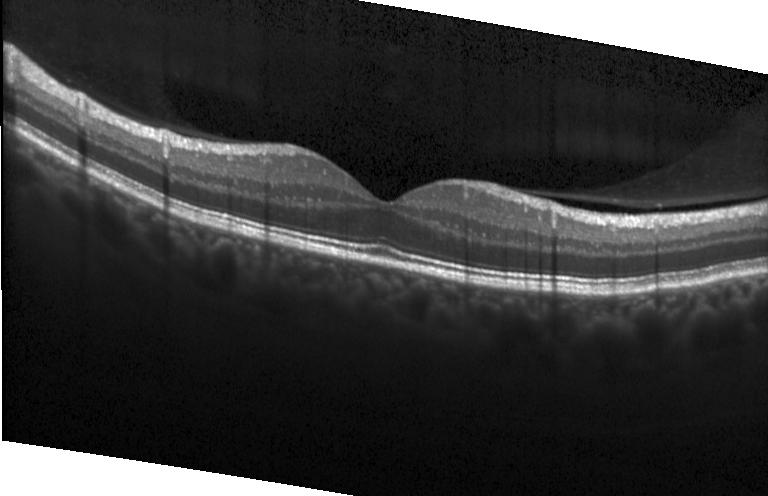
Impression: no choroidal neovascularization, no diabetic macular edema, and no drusen.